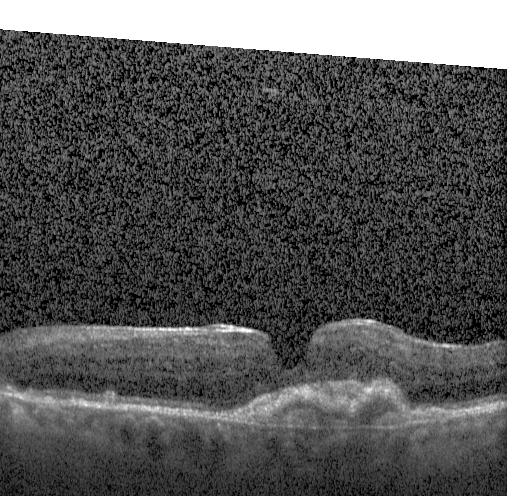
OCT finding: a choroidal neovascular membrane.